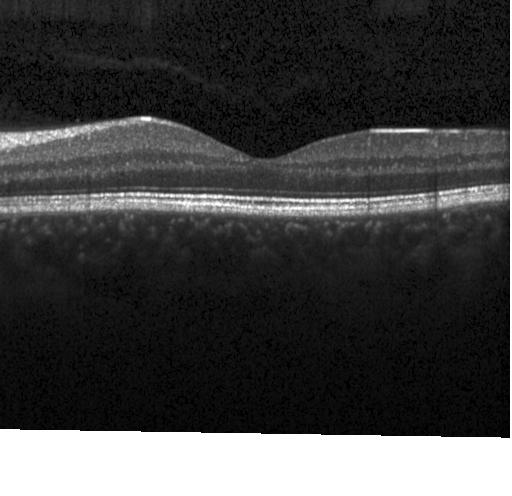 Diagnosis: no evidence of CNV, DME, or drusen.